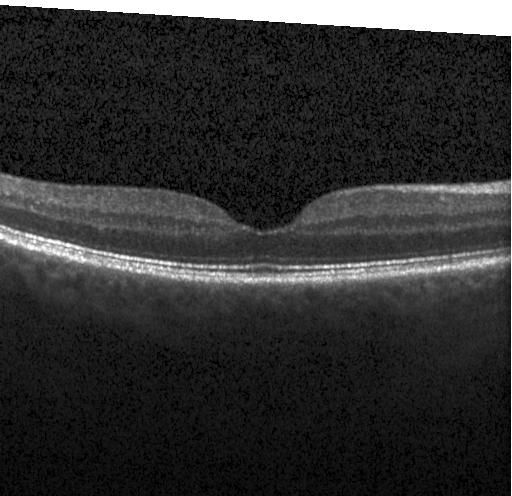

SD-OCT; optical coherence tomography scan. Macular OCT: no CNV, DME, or drusen.